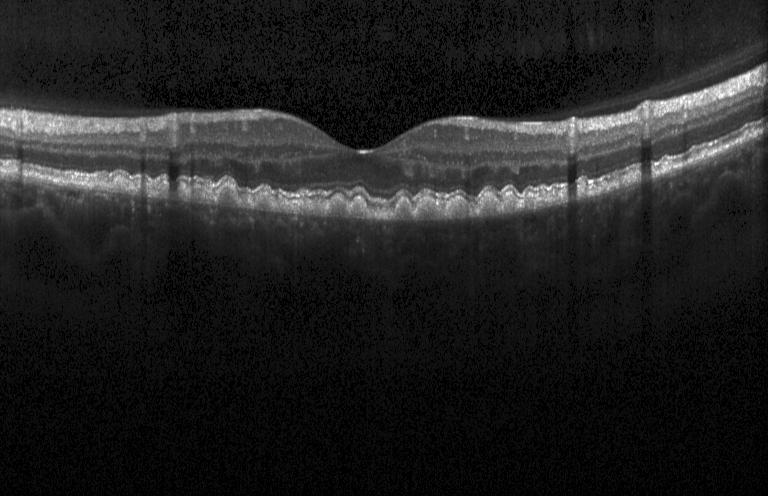 Diagnosis: sub-RPE drusenoid deposits.